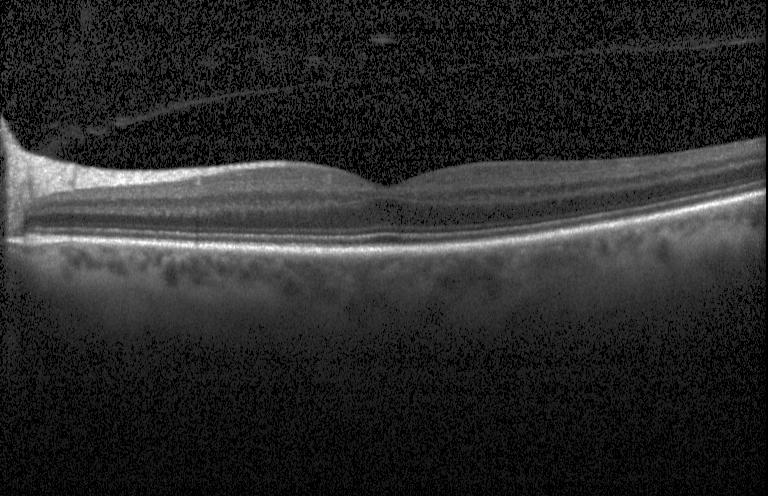

Macular OCT: no CNV, DME, or drusen.